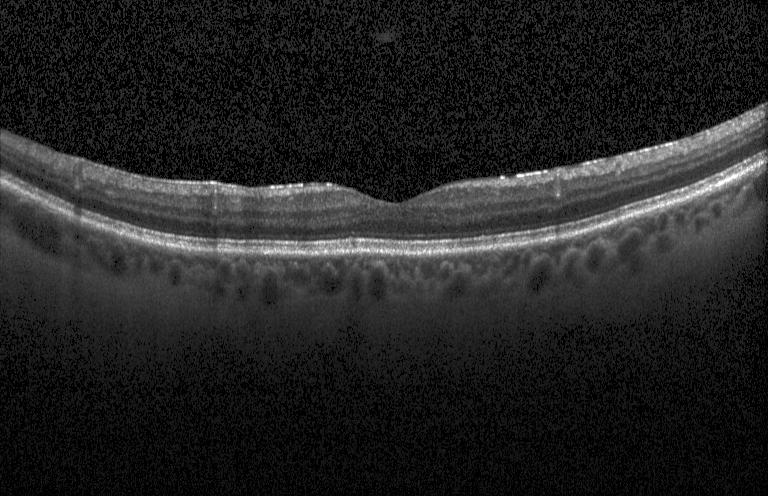 Spectral-domain OCT B-scan: no choroidal neovascularization, diabetic macular edema, or drusen.